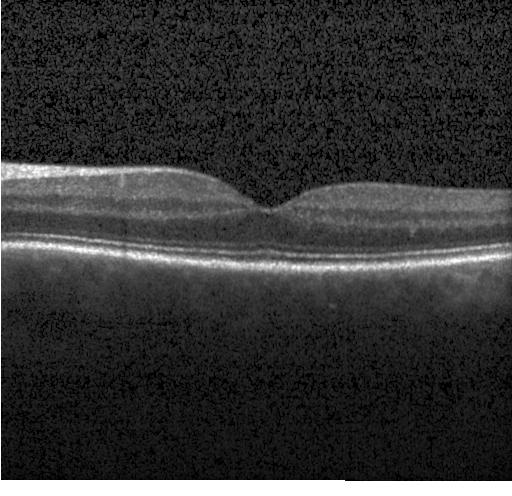

OCT B-scan — OCT finding: no CNV, no DME, and no drusen.